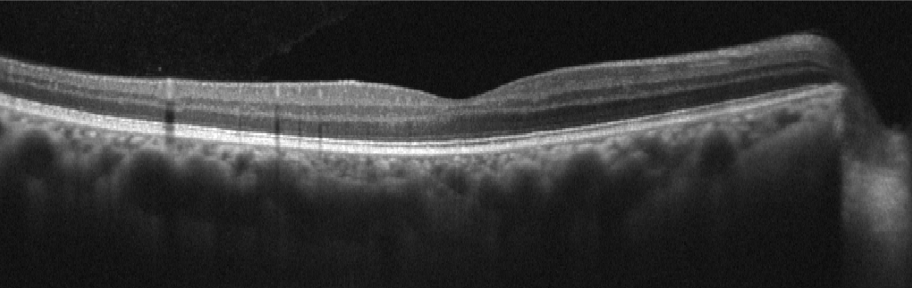 The scan shows absence of AMD, DME, ERM, RAO, RVO, and vitreomacular interface disease.